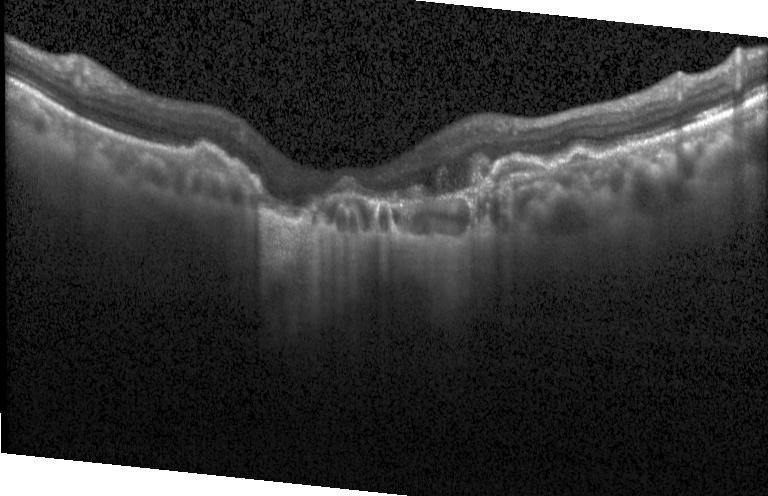 OCT B-scan showing CNV.